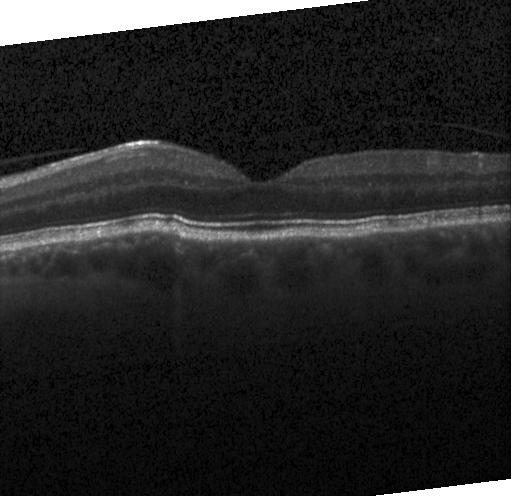

Retinal OCT cross-section. Through the macula. Finding: neither choroidal neovascularization, diabetic macular edema, nor drusen.